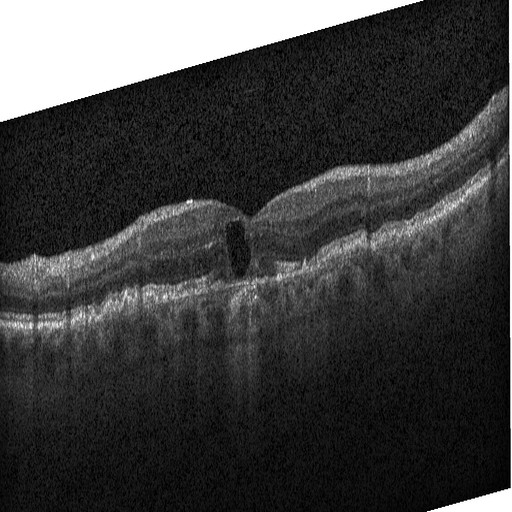

Impression: diabetic macular edema.